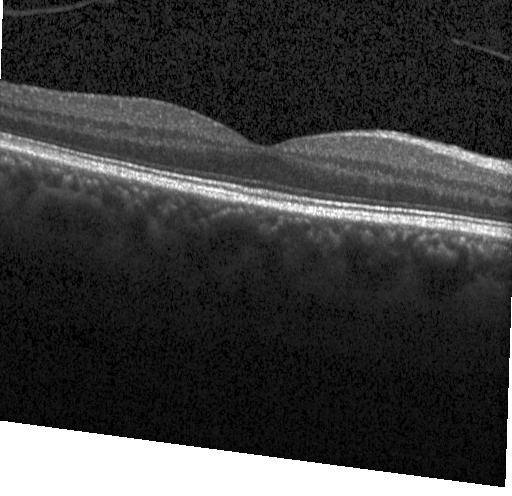

Retinal OCT B-scan — This B-scan demonstrates no evidence of choroidal neovascularization, diabetic macular edema, or drusen.